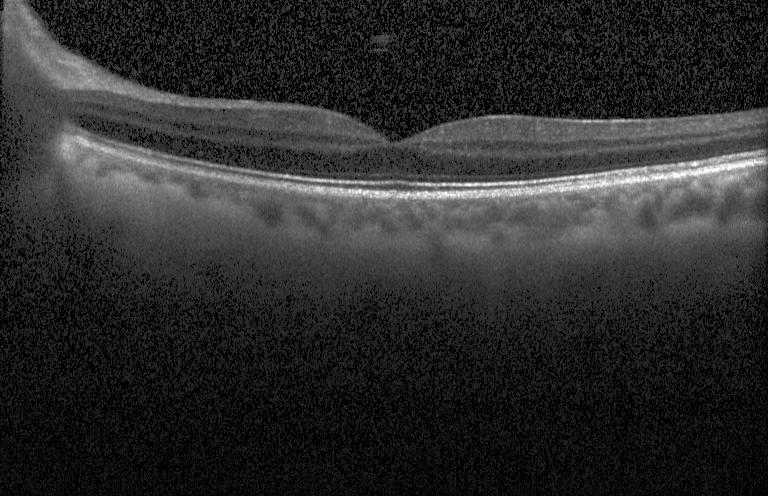
OCT line scan.
Impression: no choroidal neovascularization, no diabetic macular edema, and no drusen.